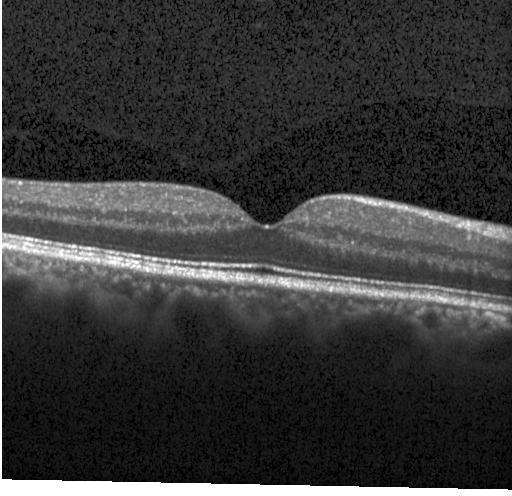 No choroidal neovascularization, diabetic macular edema, or drusen.